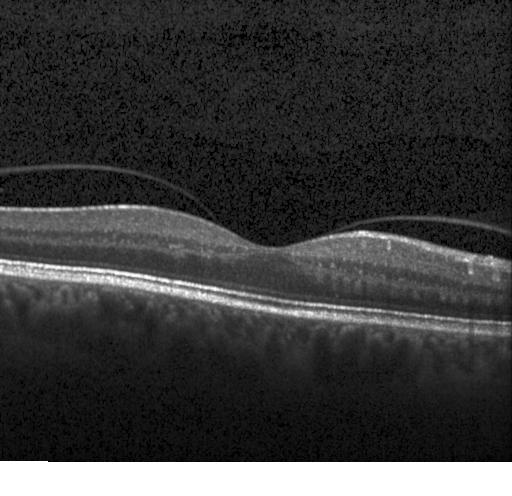 Spectral-domain OCT B-scan: no evidence of CNV, DME, or drusen.